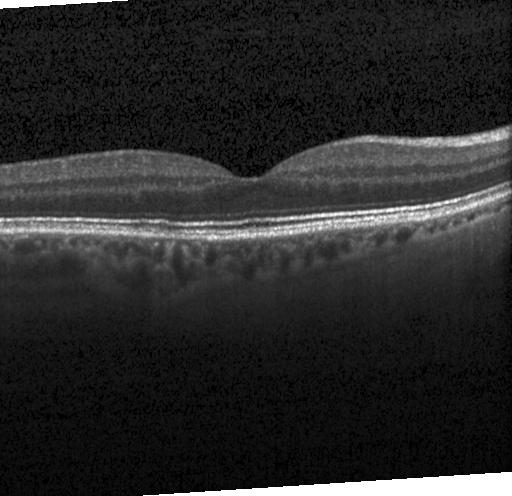 Impression: no choroidal neovascularization, diabetic macular edema, or drusen.